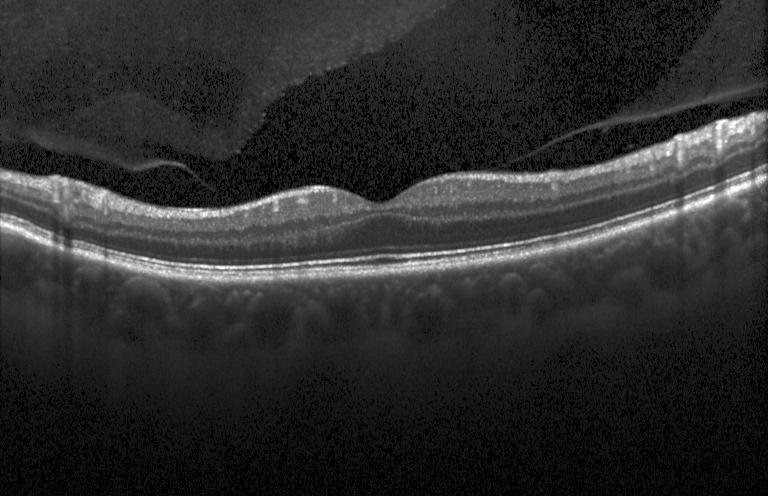
Heidelberg Spectralis OCT system. Fovea-centered. Optical coherence tomography scan.
Diagnosis: neither CNV, DME, nor drusen.